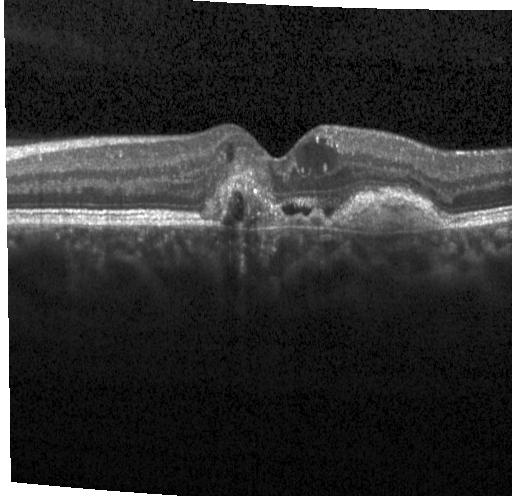
OCT scan showing choroidal neovascularization (CNV).